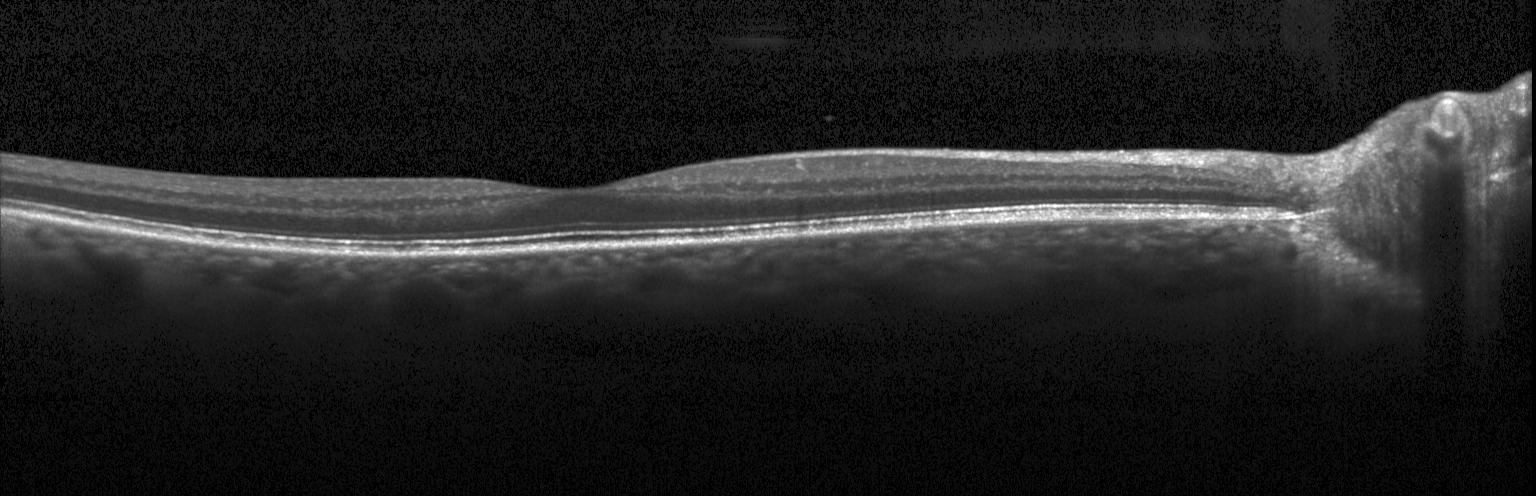

No evidence of choroidal neovascularization, diabetic macular edema, or drusen.